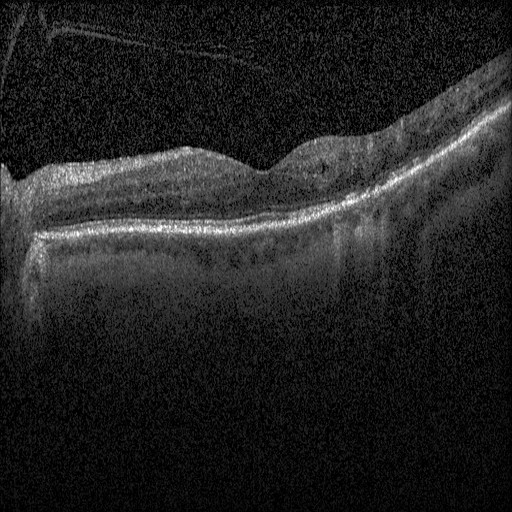 Acquired on a Heidelberg Spectralis; OCT B-scan; SD-OCT.
Macular OCT: diabetic macular edema.